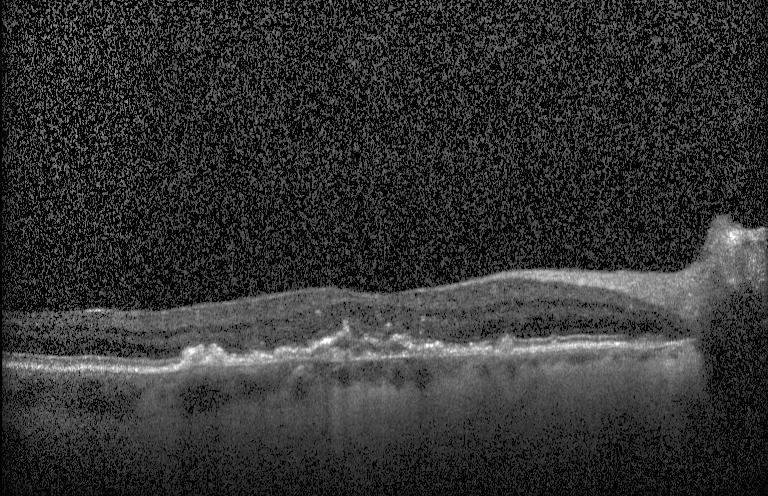
Heidelberg Spectralis OCT system · optical coherence tomography B-scan — Assessment: CNV.